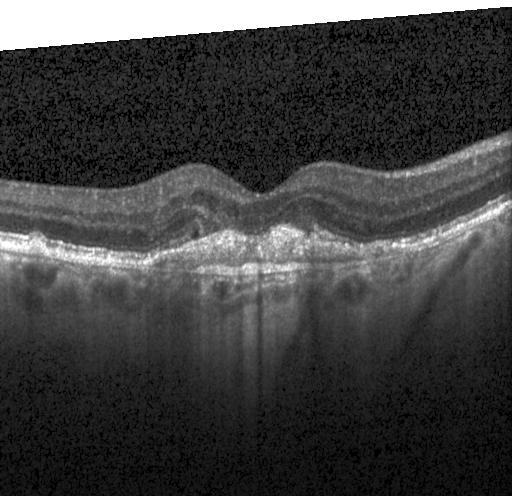 Optical coherence tomography scan. Spectral-domain OCT.
Diagnosis: a choroidal neovascular membrane.